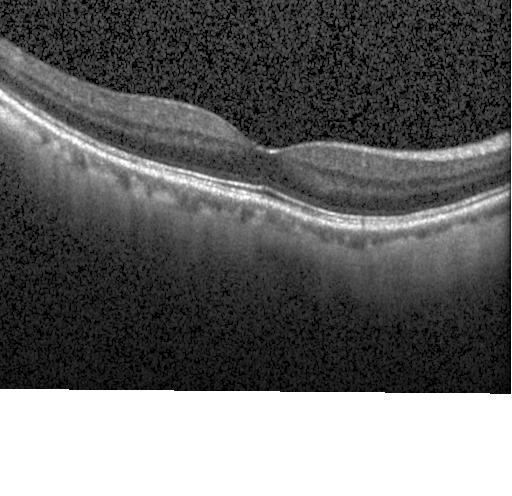 Horizontal scan through the fovea. Spectral-domain OCT. Heidelberg Spectralis. Optical coherence tomography B-scan.
This B-scan demonstrates neither CNV, DME, nor drusen.